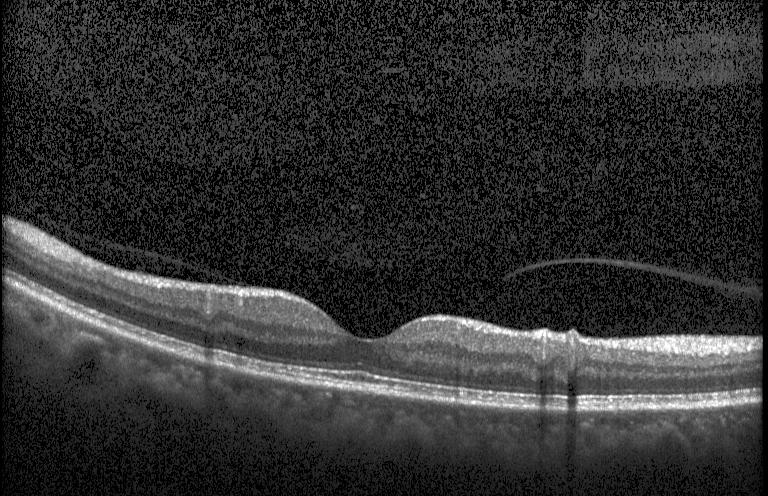

OCT line scan. Horizontal scan through the fovea
Impression: neither choroidal neovascularization, diabetic macular edema, nor drusen.